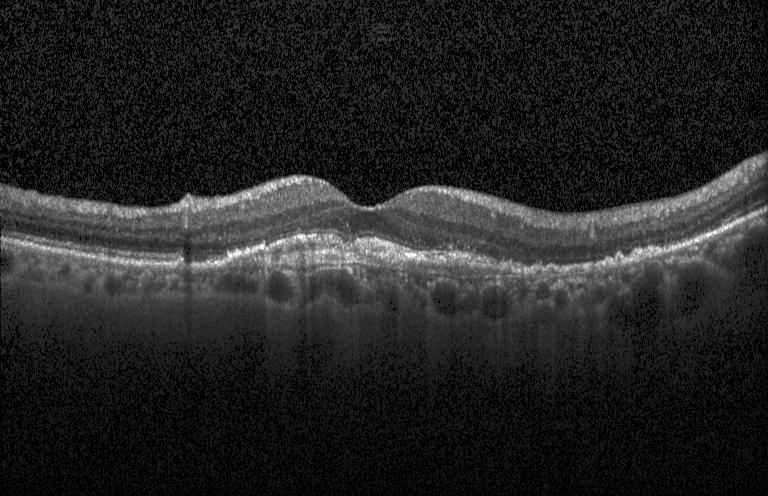

Instrument: Heidelberg Spectralis · horizontal scan through the fovea · OCT B-scan
Diagnosis: a choroidal neovascular membrane.